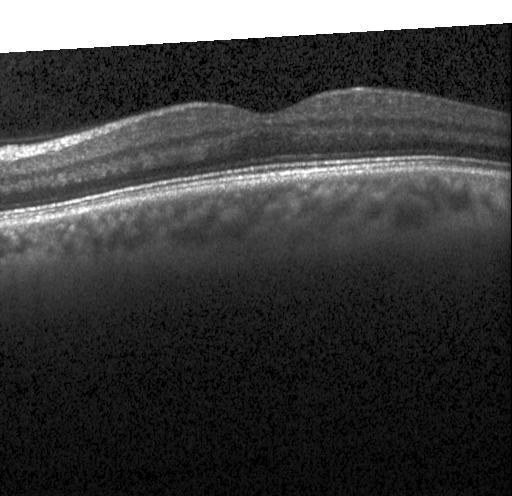
Dx: no evidence of choroidal neovascularization, diabetic macular edema, or drusen.